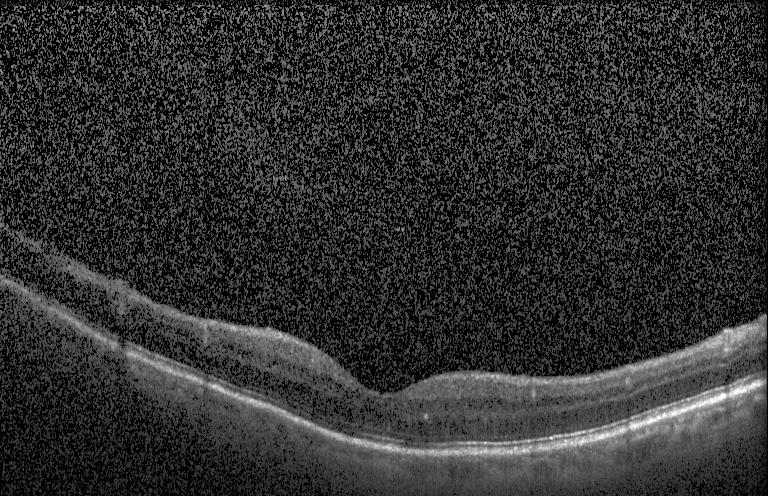

Dx: neither CNV, DME, nor drusen.